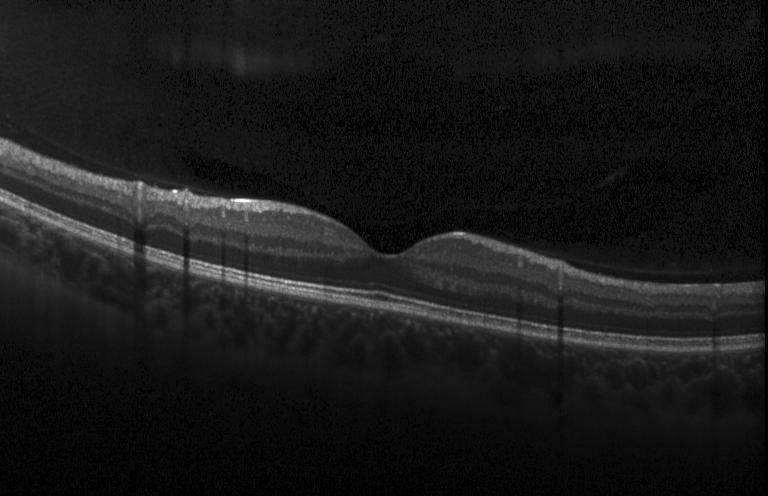 Assessment: no evidence of CNV, DME, or drusen.